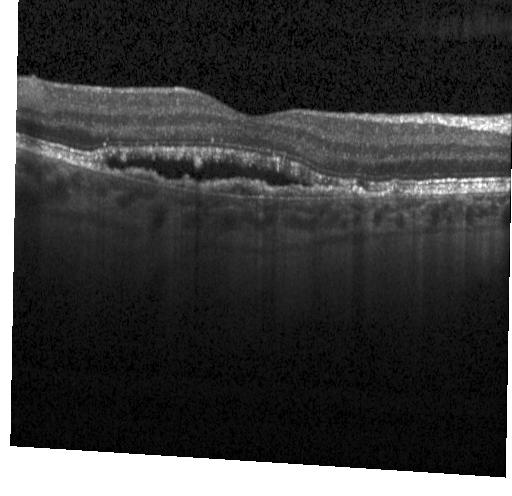 Dx: choroidal neovascularization.